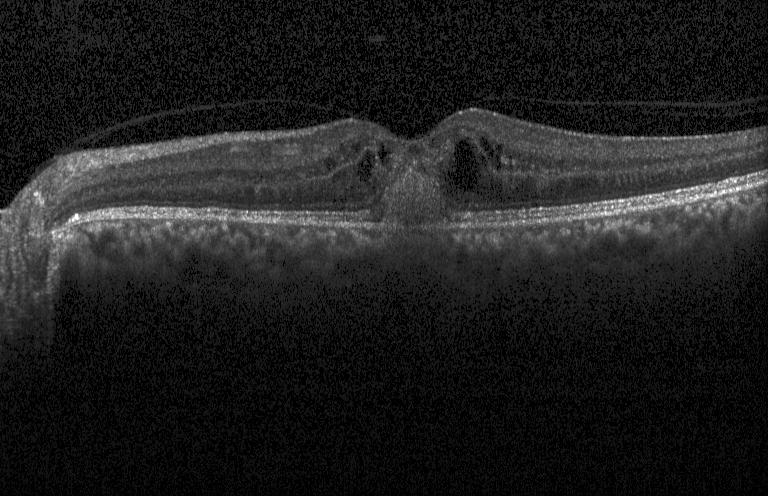

OCT line scan; spectral-domain OCT.
Dx: a choroidal neovascular membrane.